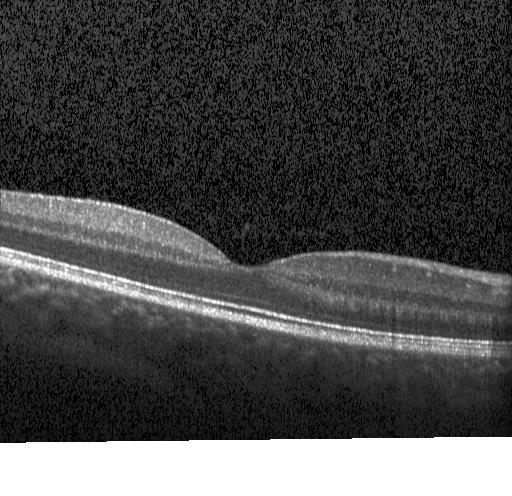 Spectral-domain optical coherence tomography · horizontal scan through the fovea · OCT line scan · Heidelberg Spectralis OCT system
Impression: neither CNV, DME, nor drusen.